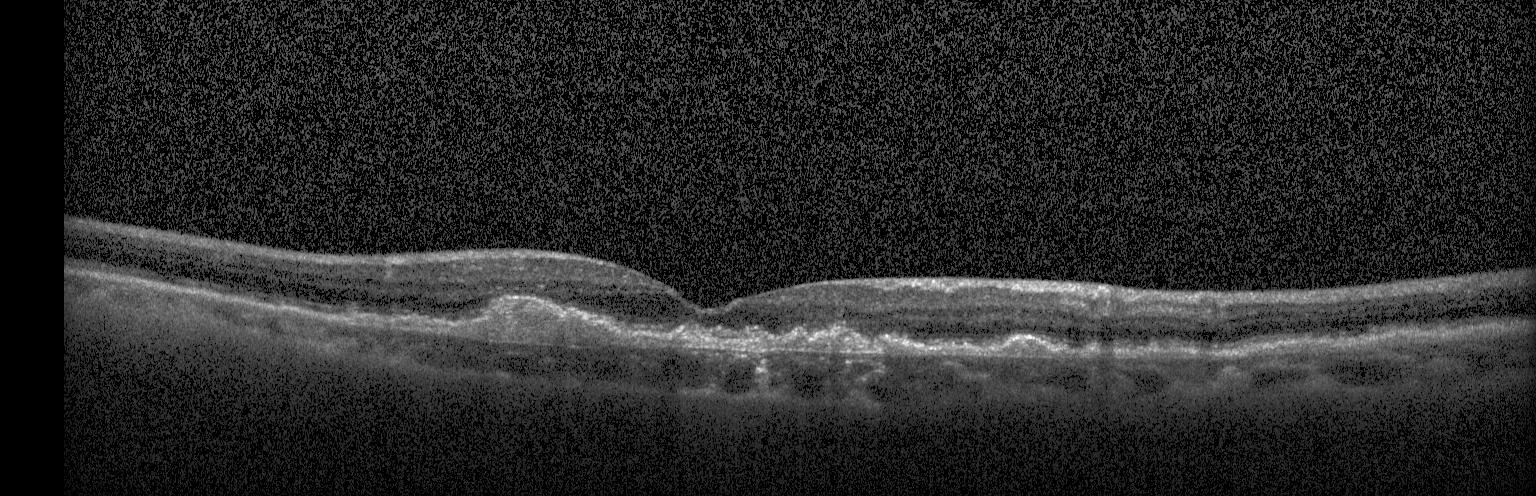
Through the macula; acquired on a Heidelberg Spectralis; OCT line scan; spectral-domain optical coherence tomography — The scan shows a choroidal neovascular membrane.